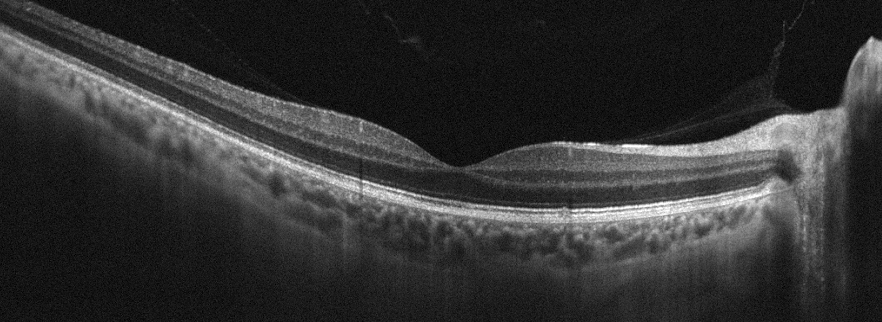 Macular scan; acquired on an Optovue Avanti RTVue XR; OD; OCT line scan — The scan shows no evidence of AMD, DME, ERM, RAO, RVO, or VID.